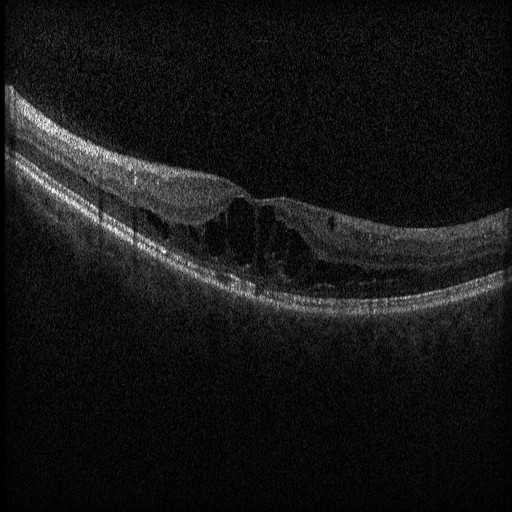 Diagnosis: DME.